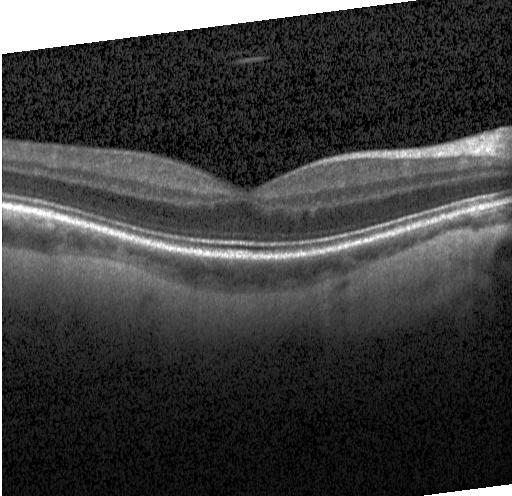

Diagnosis: no evidence of choroidal neovascularization, diabetic macular edema, or drusen.